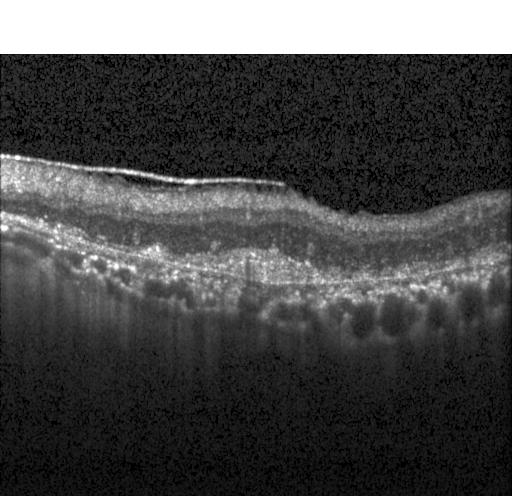
Choroidal neovascularization (CNV).